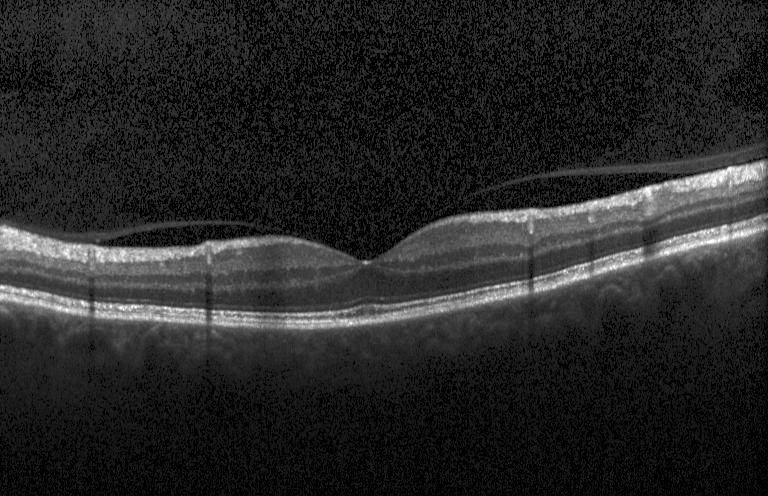

Diagnosis: neither choroidal neovascularization, diabetic macular edema, nor drusen.